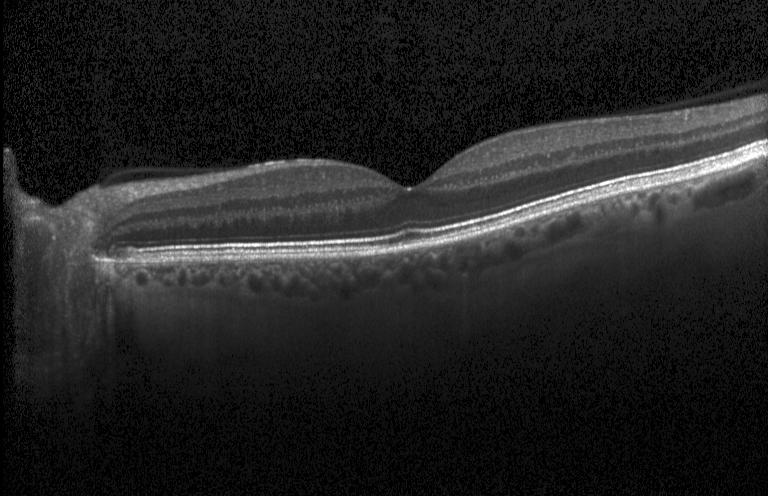

Finding: no choroidal neovascularization, diabetic macular edema, or drusen.